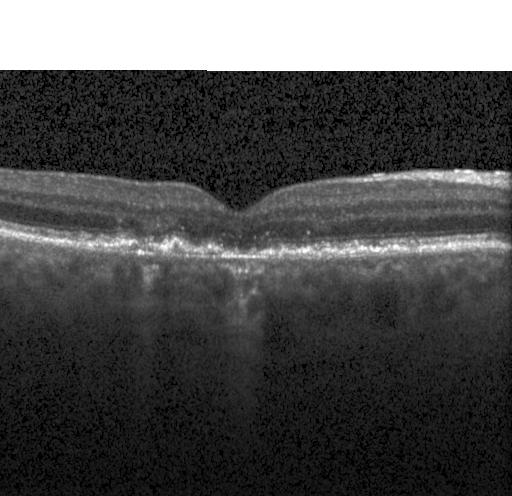 OCT line scan — Impression: a choroidal neovascular membrane.